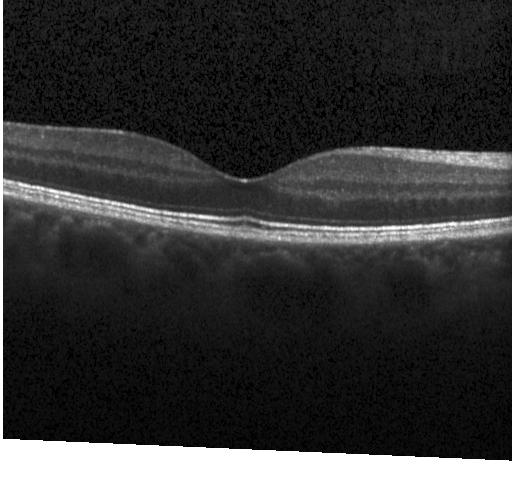

Diagnosis: no evidence of choroidal neovascularization, diabetic macular edema, or drusen.